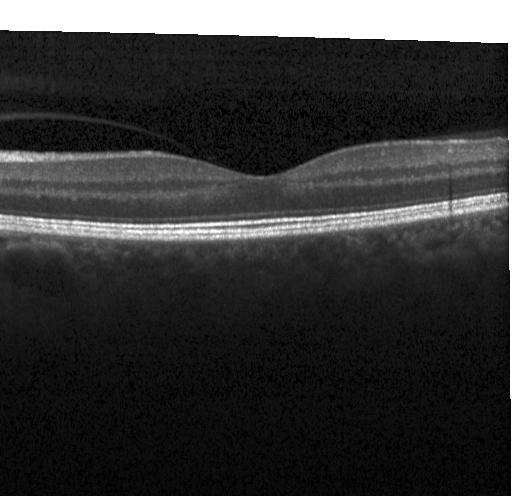

Optical coherence tomography B-scan · spectral-domain optical coherence tomography · centered on the fovea — OCT finding: no evidence of choroidal neovascularization, diabetic macular edema, or drusen.